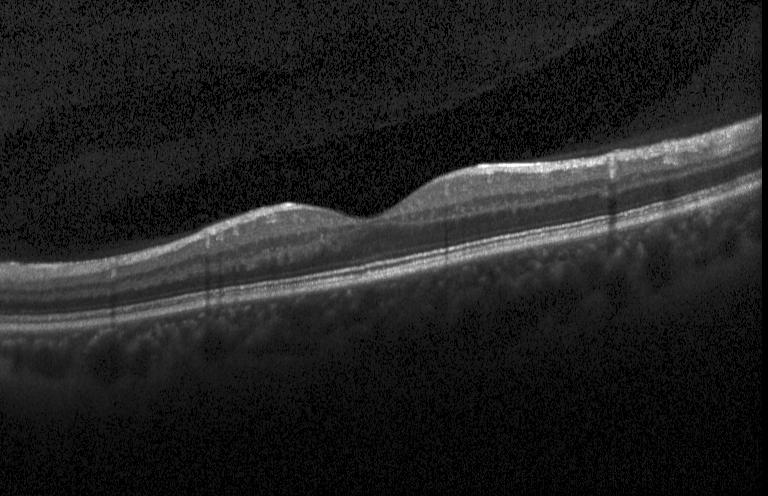

Retinal OCT B-scan; SD-OCT — The scan shows no choroidal neovascularization, no diabetic macular edema, and no drusen.